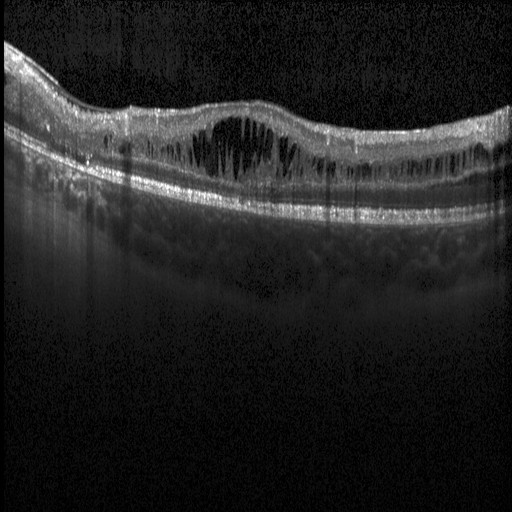

Diagnosis: DME.